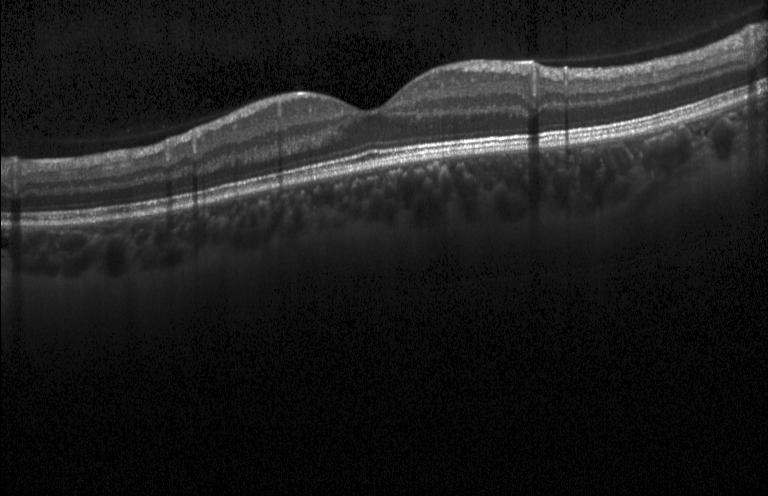 Macular OCT: neither choroidal neovascularization, diabetic macular edema, nor drusen.